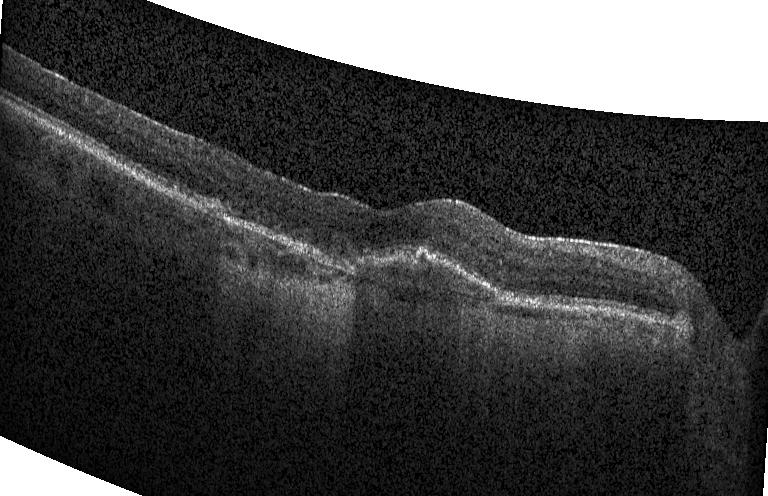
SD-OCT. Centered on the fovea. Optical coherence tomography scan. Acquired on a Heidelberg Spectralis. Diagnosis: a choroidal neovascular membrane.